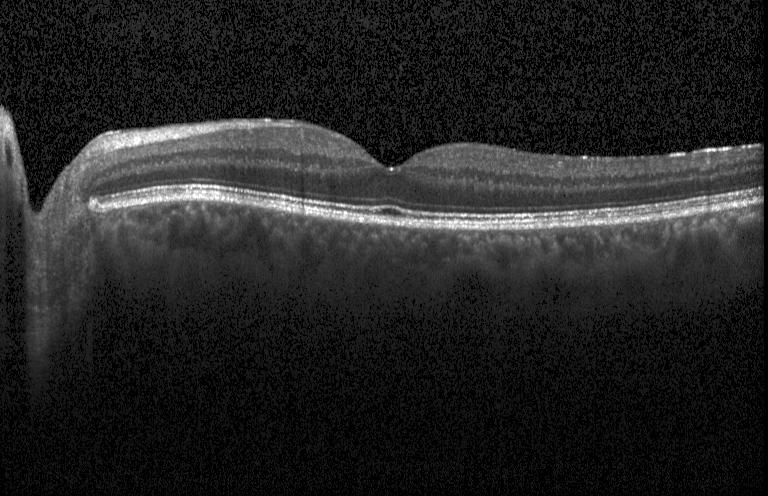

Instrument: Heidelberg Spectralis, retinal OCT cross-section, fovea-centered. The scan shows no choroidal neovascularization, no diabetic macular edema, and no drusen.